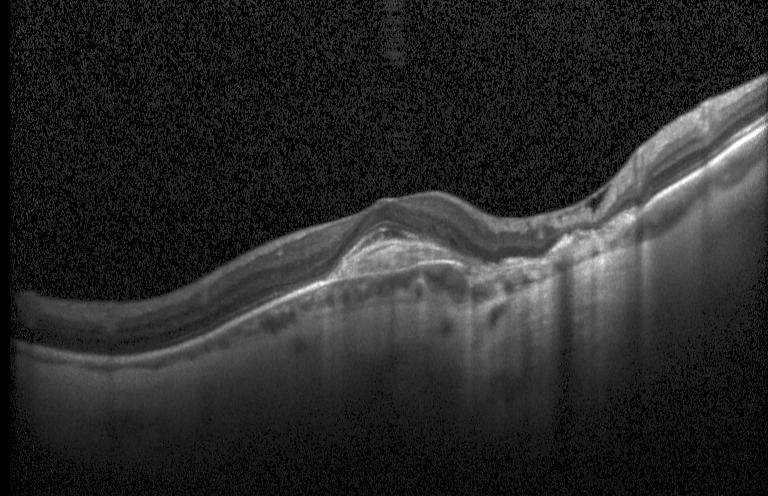
OCT scan showing choroidal neovascularization.